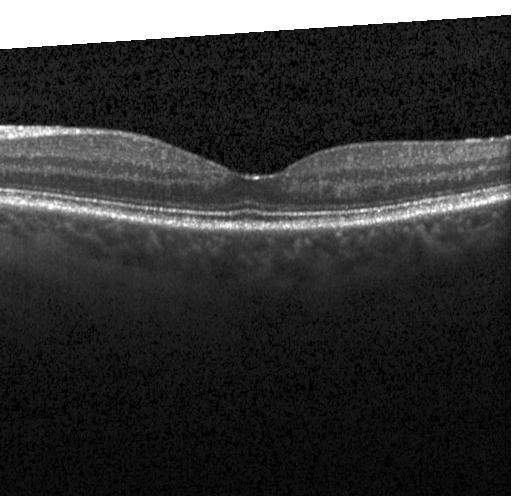
Dx: no CNV, no DME, and no drusen.